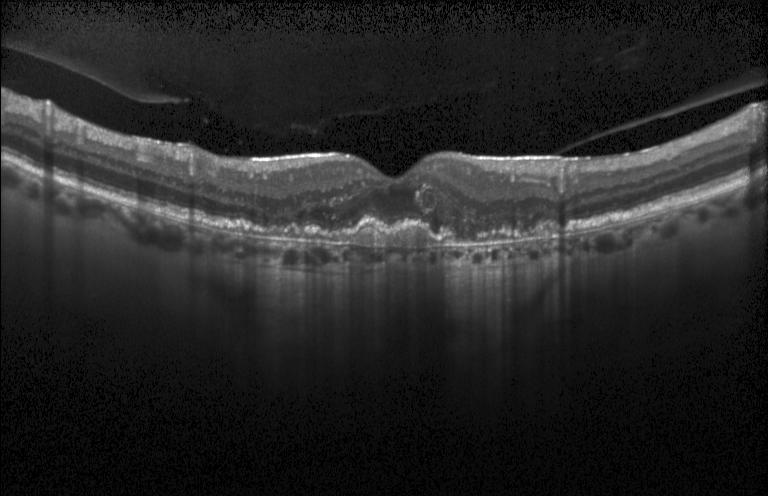 Finding: a choroidal neovascular membrane.